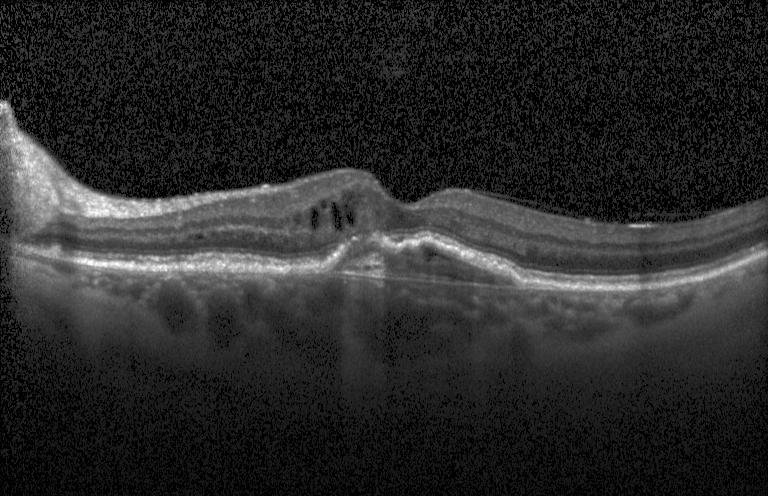 Centered on the fovea · optical coherence tomography B-scan.
This B-scan demonstrates a choroidal neovascular membrane.